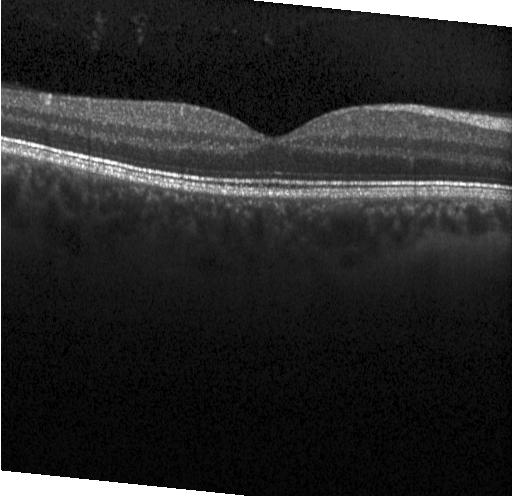 Dx: no choroidal neovascularization, no diabetic macular edema, and no drusen.